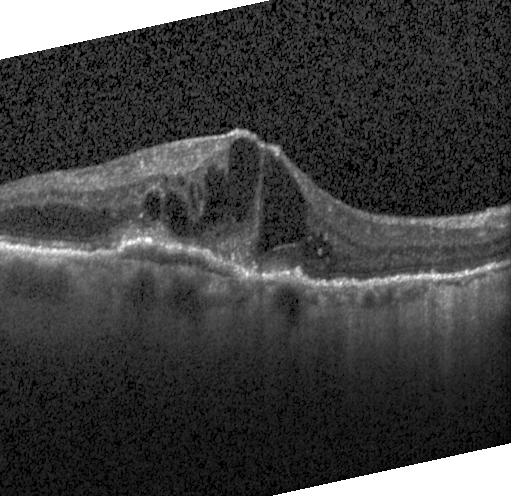
Spectral-domain optical coherence tomography; through the macula; optical coherence tomography B-scan; instrument: Heidelberg Spectralis.
Finding: a choroidal neovascular membrane.